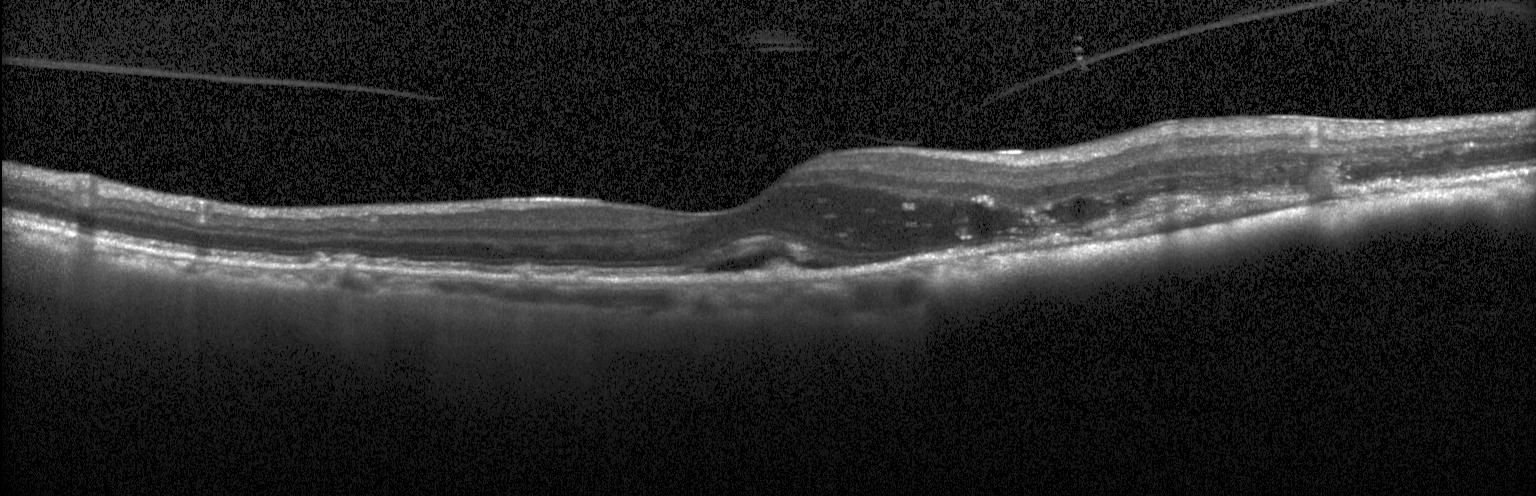 Optical coherence tomography B-scan
Finding: CNV.